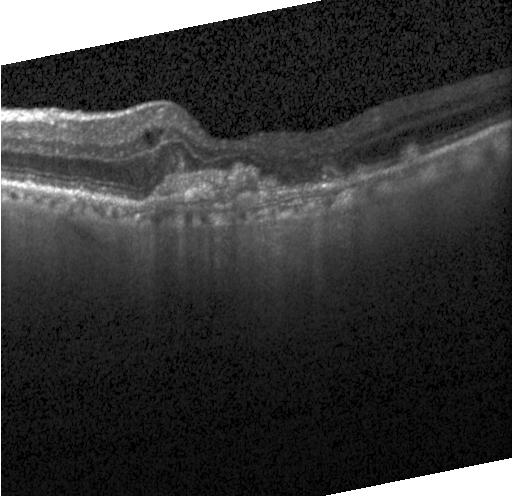
Retinal OCT B-scan. Dx: CNV.